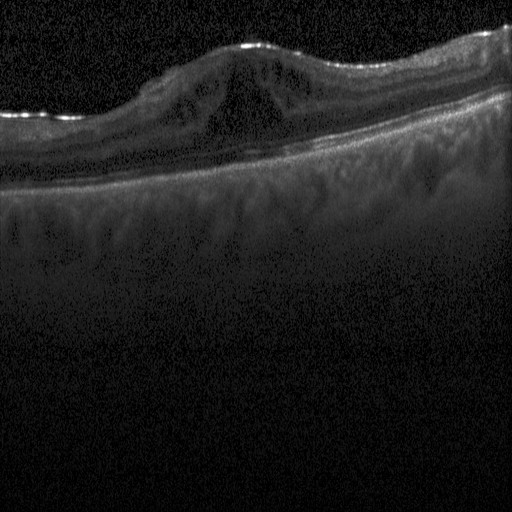 Centered on the fovea · SD-OCT · OCT line scan — This B-scan demonstrates DME.